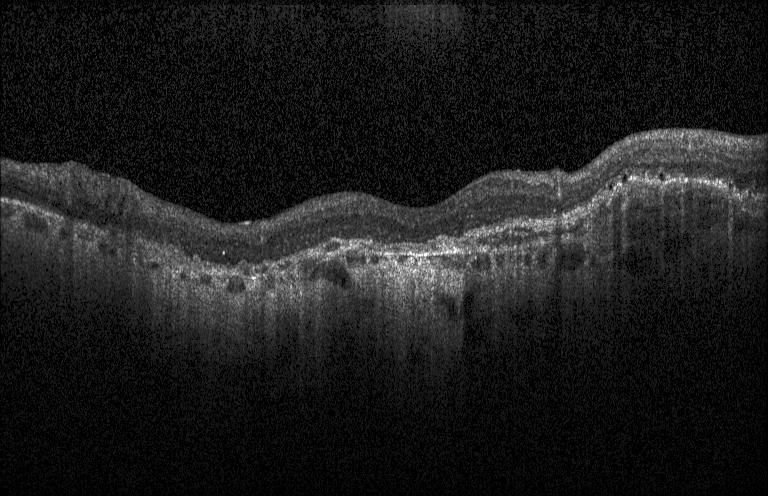 Heidelberg Spectralis OCT system · OCT line scan.
Macular OCT: a choroidal neovascular membrane.